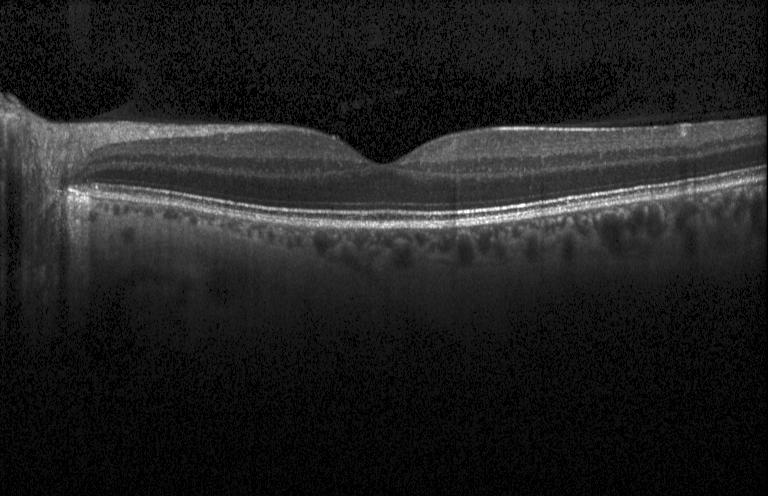 Retinal OCT cross-section · macular scan.
Finding: neither choroidal neovascularization, diabetic macular edema, nor drusen.